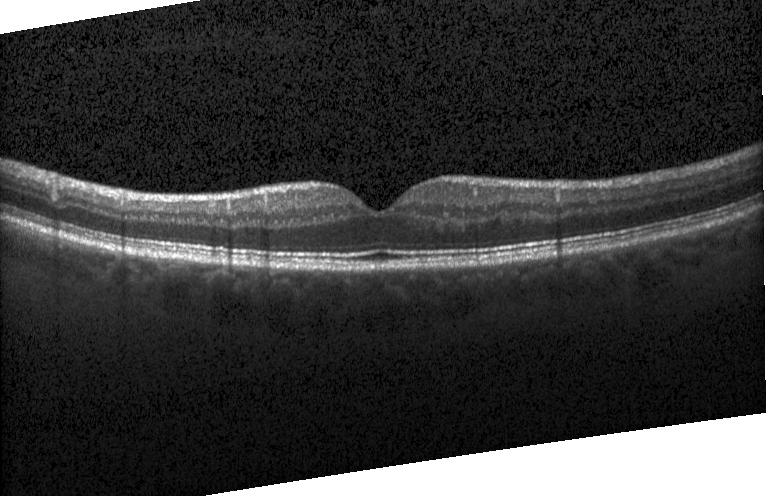 Retinal OCT cross-section; spectral-domain optical coherence tomography. Impression: no choroidal neovascularization, no diabetic macular edema, and no drusen.